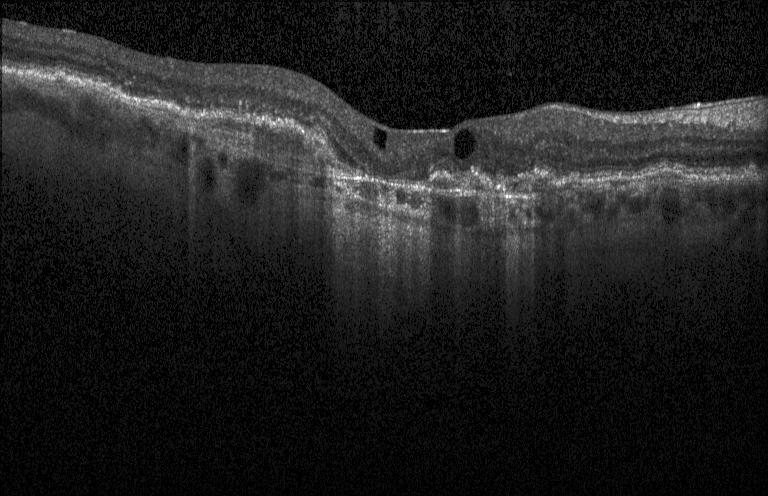

OCT line scan, centered on the fovea, spectral-domain optical coherence tomography
Dx: a choroidal neovascular membrane.